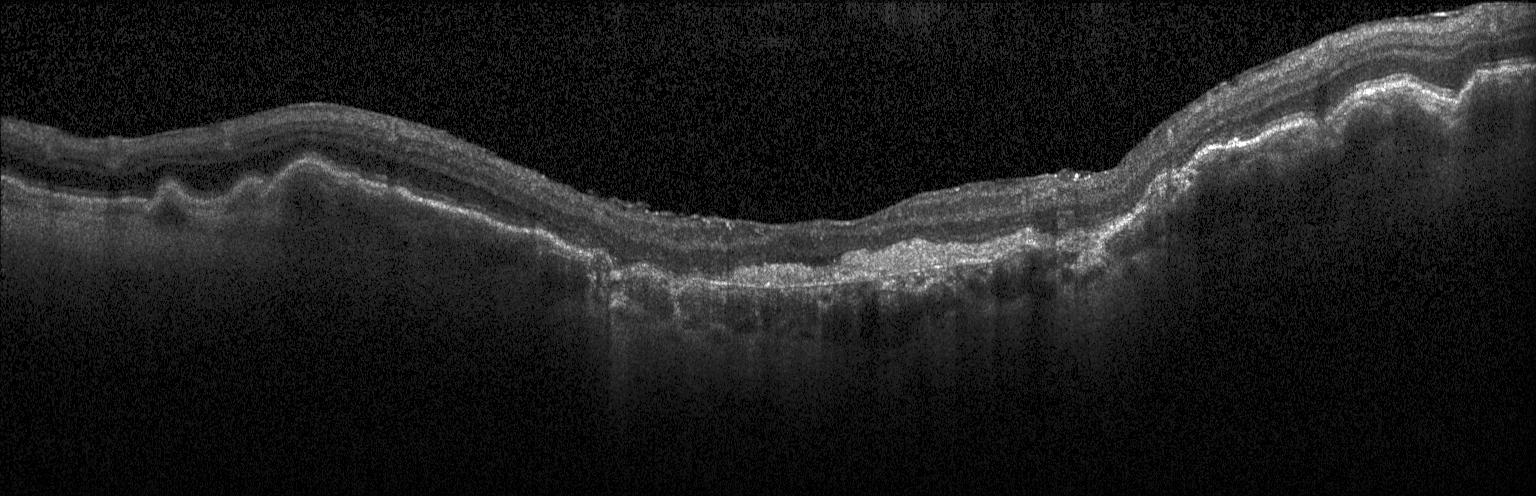 Macular OCT demonstrating CNV.